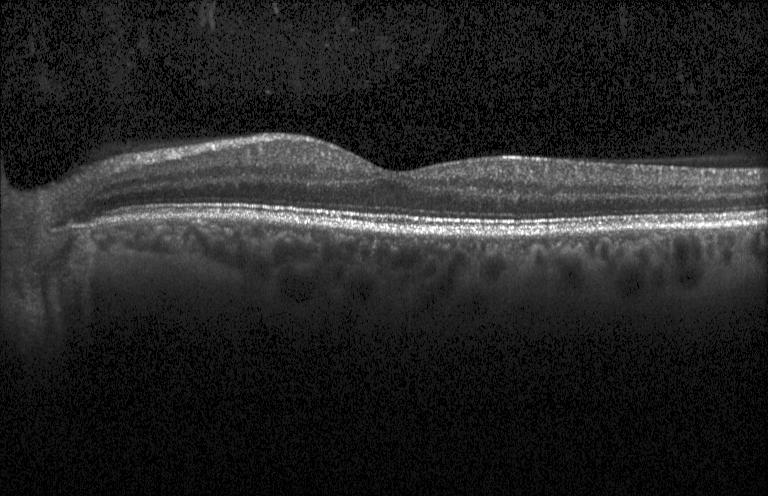
Impression: no choroidal neovascularization, no diabetic macular edema, and no drusen.